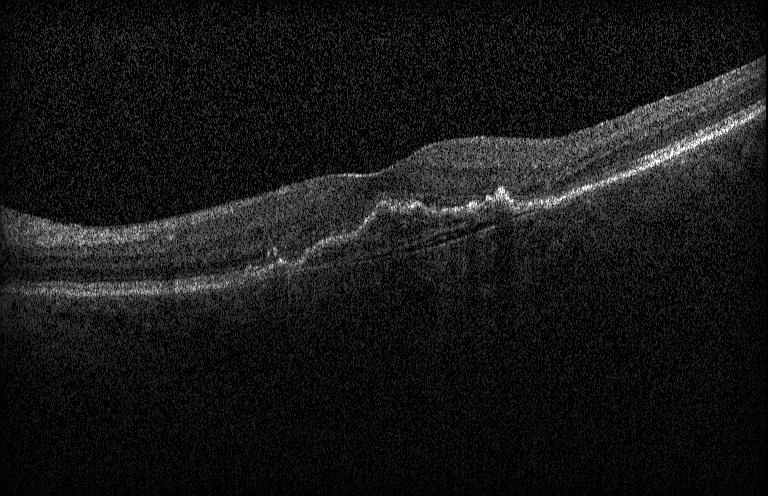
Spectral-domain OCT, optical coherence tomography B-scan. This B-scan demonstrates a choroidal neovascular membrane.